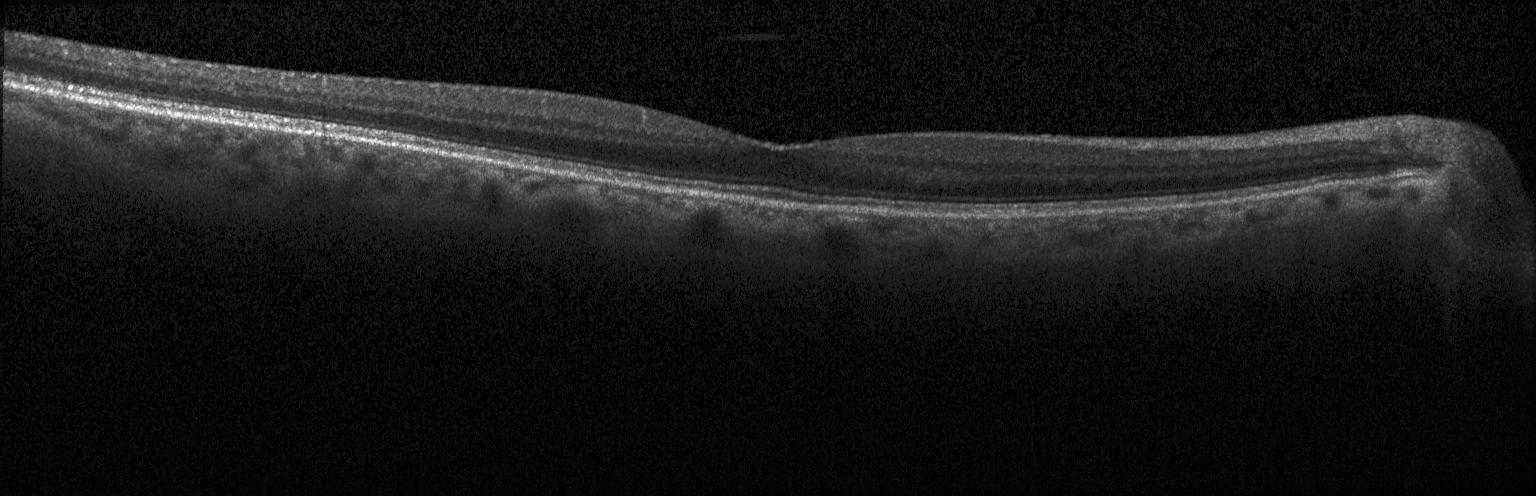 Retinal OCT cross-section showing neither choroidal neovascularization, diabetic macular edema, nor drusen.